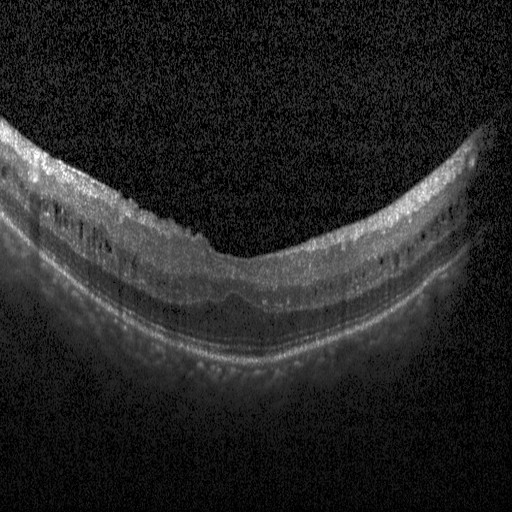

This B-scan demonstrates diabetic macular edema (DME).